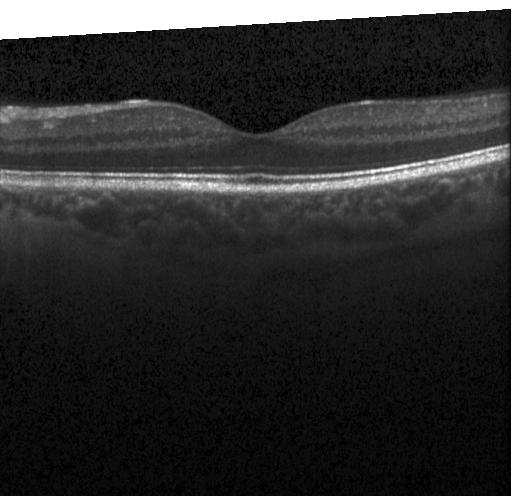 Macular scan · optical coherence tomography B-scan · spectral-domain optical coherence tomography.
Diagnosis: no choroidal neovascularization, no diabetic macular edema, and no drusen.